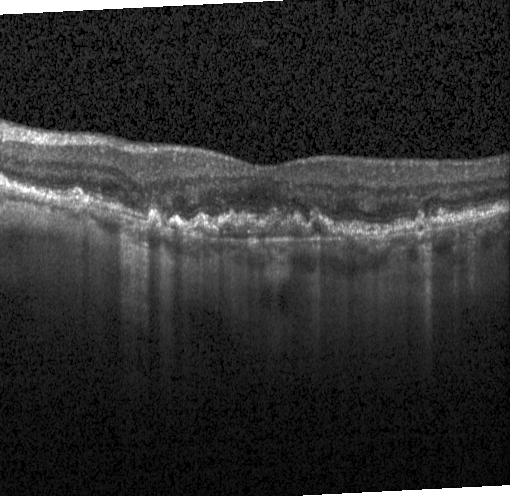
Diagnosis: choroidal neovascularization (CNV).